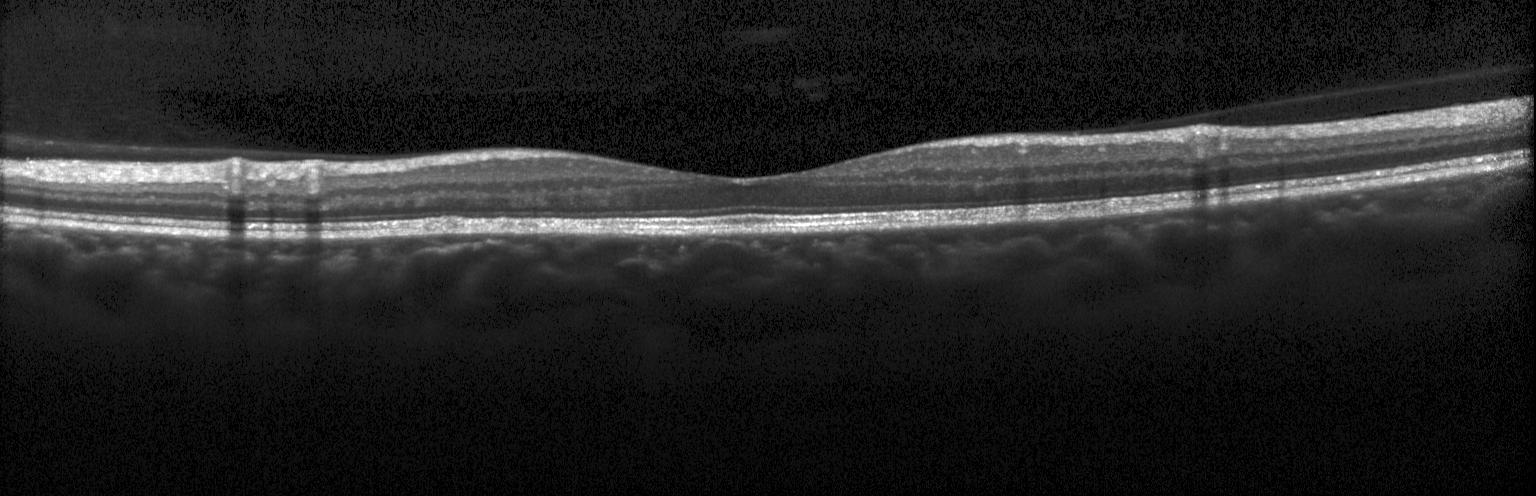 Optical coherence tomography B-scan. Acquired on a Heidelberg Spectralis. SD-OCT.
Dx: neither CNV, DME, nor drusen.